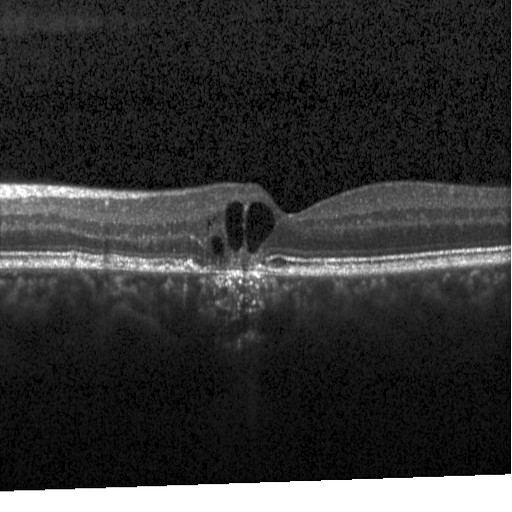

OCT line scan. Macular OCT: diabetic macular edema (DME).